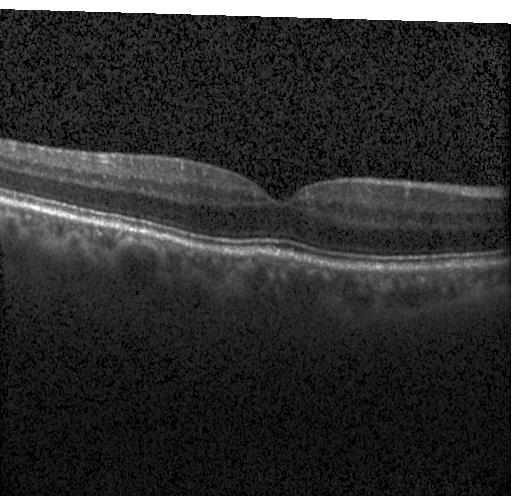
Impression: neither choroidal neovascularization, diabetic macular edema, nor drusen.